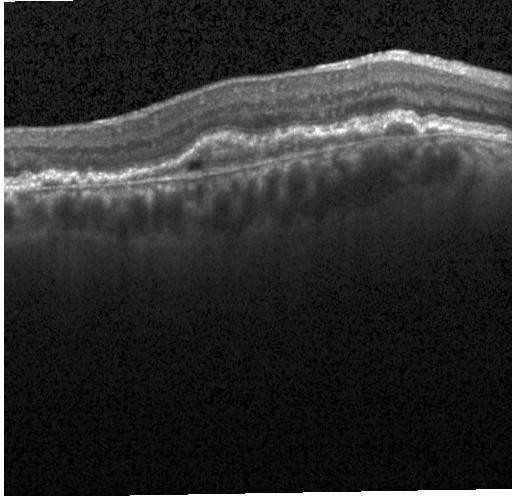
Acquired on a Heidelberg Spectralis. Retinal OCT B-scan. SD-OCT. Diagnosis: a choroidal neovascular membrane.